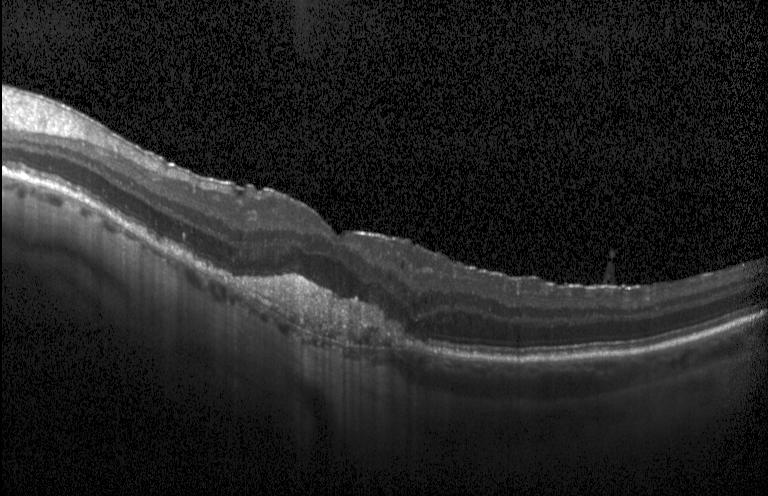
SD-OCT · retinal OCT B-scan · Heidelberg Spectralis OCT system · macular scan. Diagnosis: CNV.